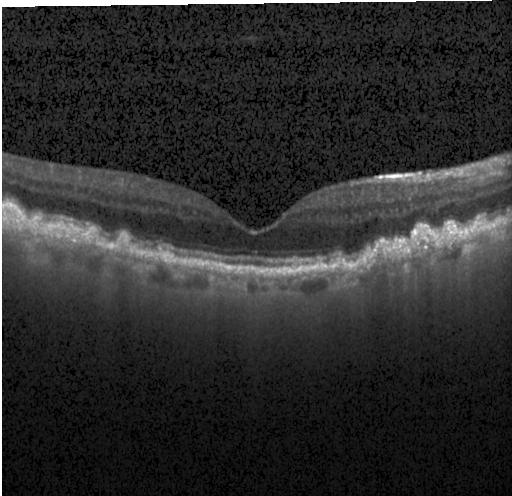
Impression: multiple drusen.